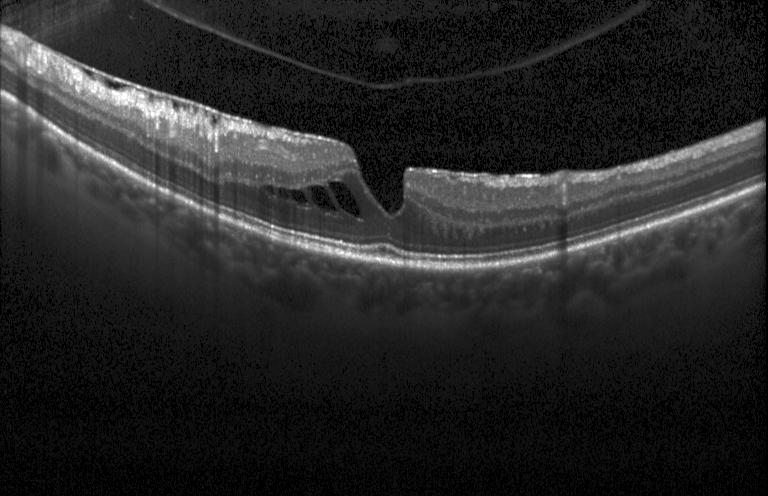

OCT B-scan. Spectral-domain OCT. Heidelberg Spectralis OCT system.
Finding: diabetic macular edema.